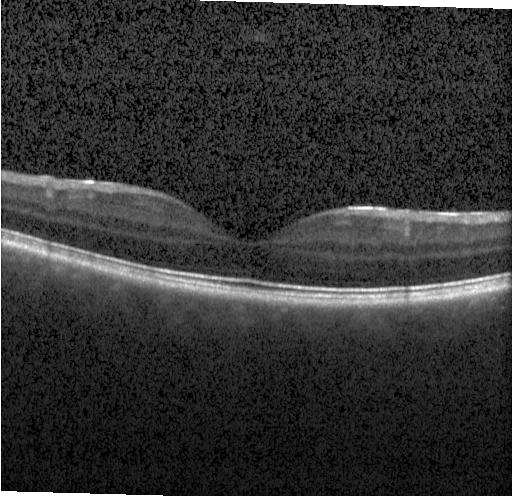
The scan shows no CNV, no DME, and no drusen.